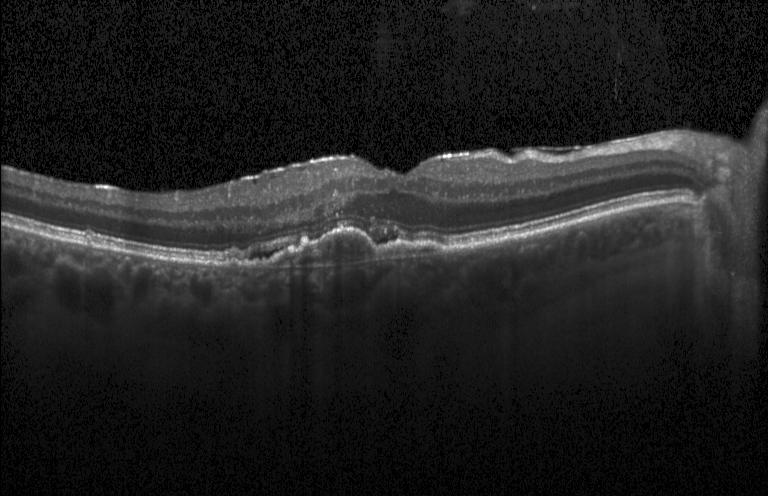

OCT scan showing choroidal neovascularization.